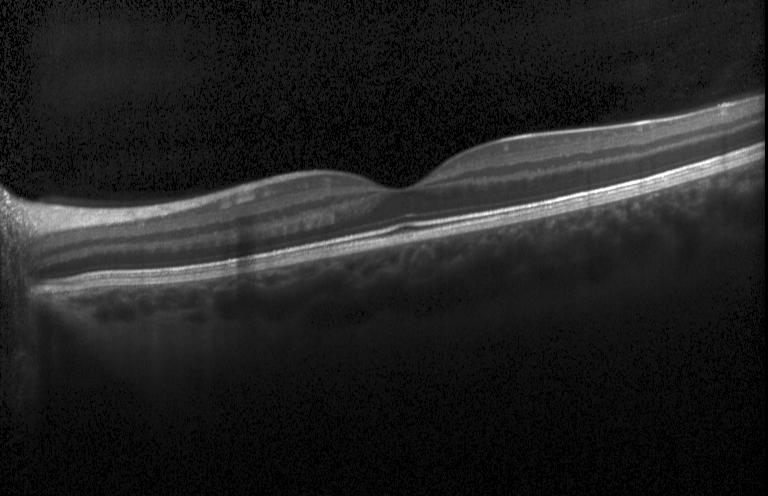 Spectral-domain OCT. Heidelberg Spectralis OCT system. Horizontal scan through the fovea. OCT B-scan
Finding: no choroidal neovascularization, diabetic macular edema, or drusen.